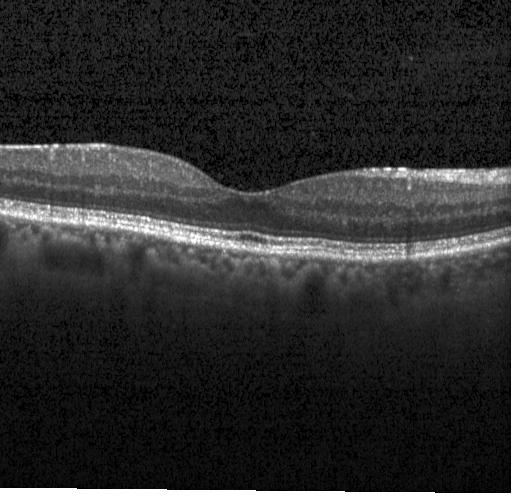 Spectral-domain OCT B-scan: neither CNV, DME, nor drusen.